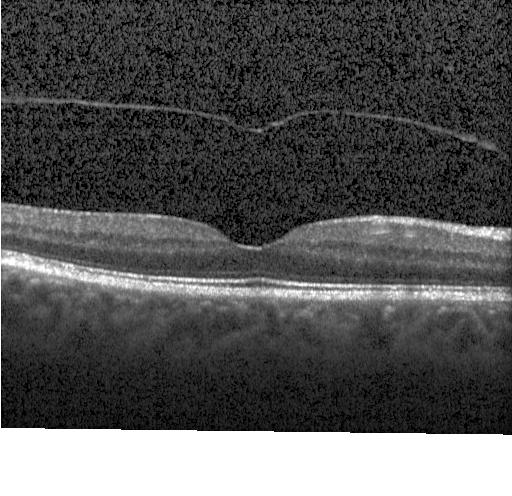

Optical coherence tomography scan
Diagnosis: no choroidal neovascularization, diabetic macular edema, or drusen.